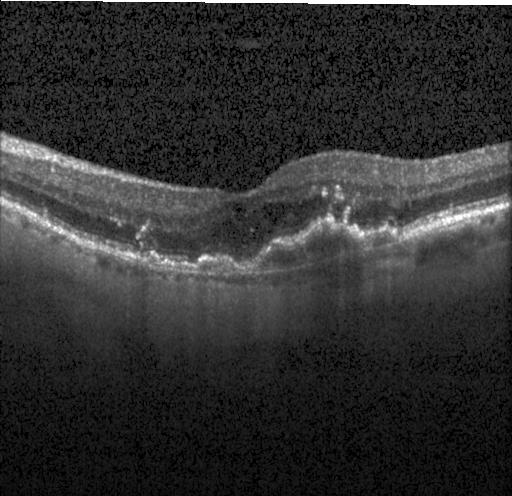
Spectral-domain OCT B-scan: a choroidal neovascular membrane.